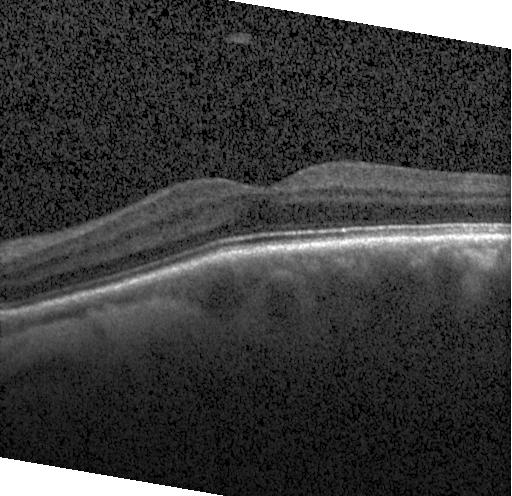
Heidelberg Spectralis OCT system; retinal OCT B-scan; through the macula; spectral-domain OCT. Diagnosis: no choroidal neovascularization, no diabetic macular edema, and no drusen.